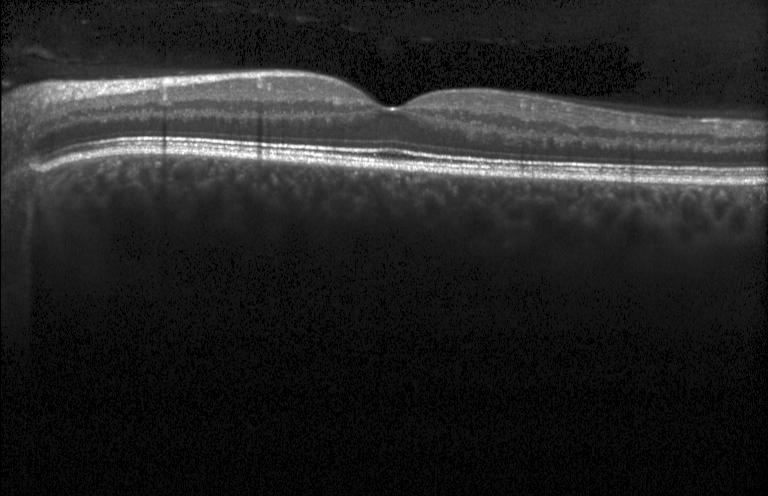 Optical coherence tomography scan; Heidelberg Spectralis.
Finding: no choroidal neovascularization, diabetic macular edema, or drusen.